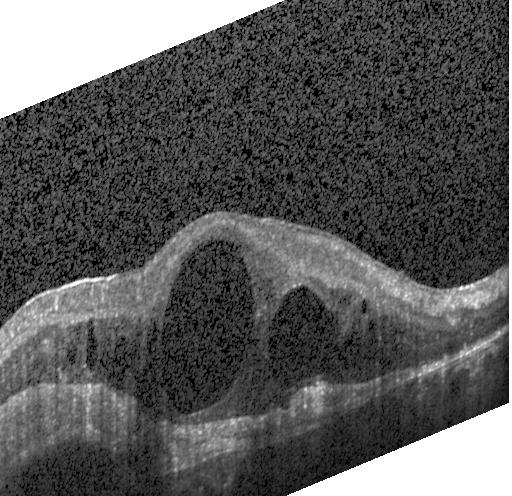

OCT line scan; macular scan — Impression: choroidal neovascularization.